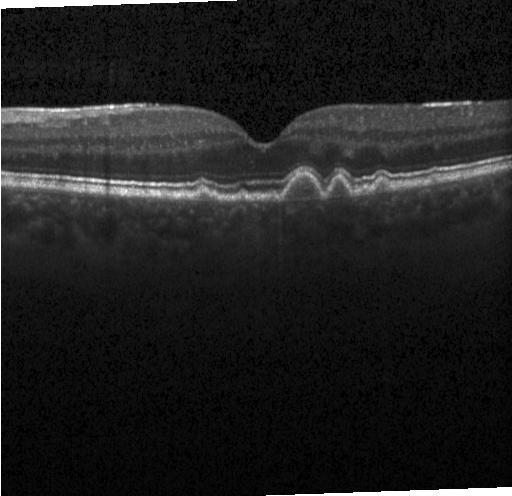
OCT line scan, macular scan, instrument: Heidelberg Spectralis
Impression: sub-RPE drusenoid deposits.